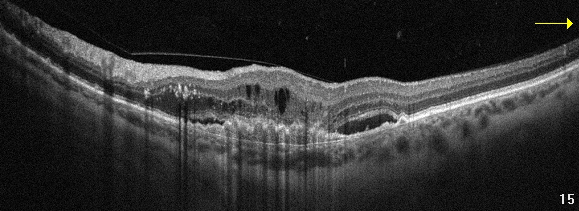 OCT line scan — Diagnosis: age-related macular degeneration (AMD).